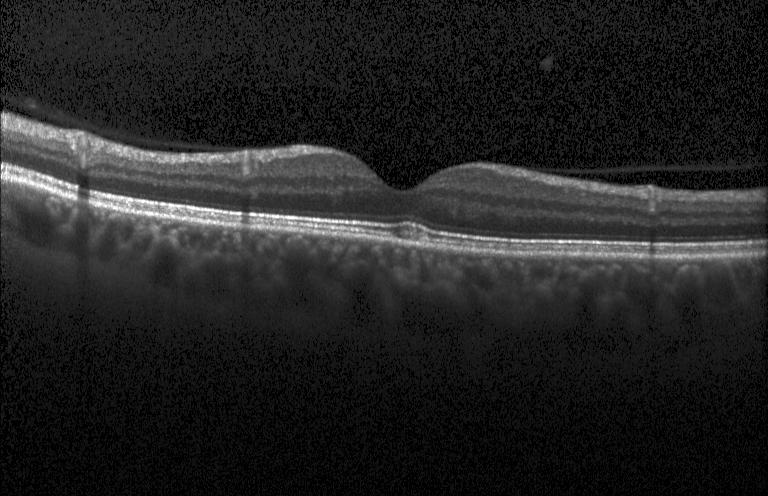

No evidence of choroidal neovascularization, diabetic macular edema, or drusen.